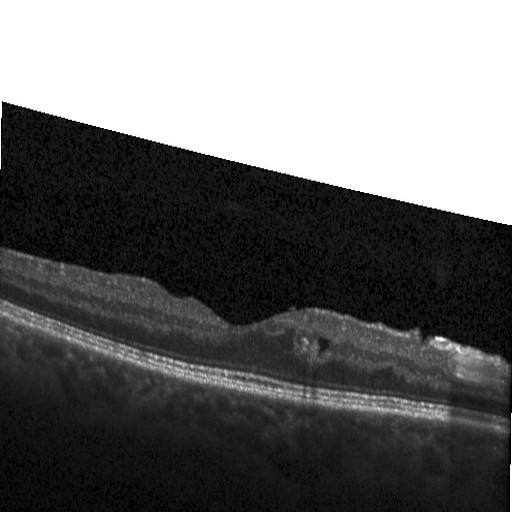
Macular OCT demonstrating DME.